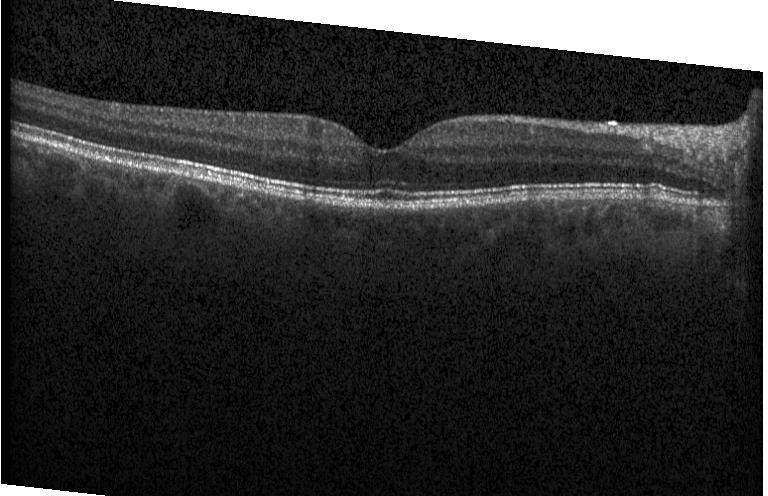 Retinal OCT cross-section.
Impression: no evidence of choroidal neovascularization, diabetic macular edema, or drusen.